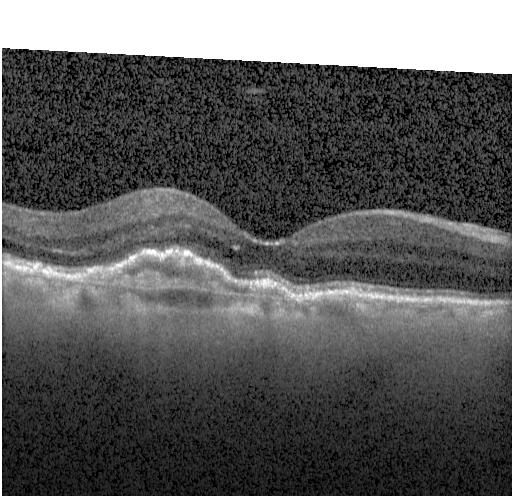
This B-scan demonstrates choroidal neovascularization.